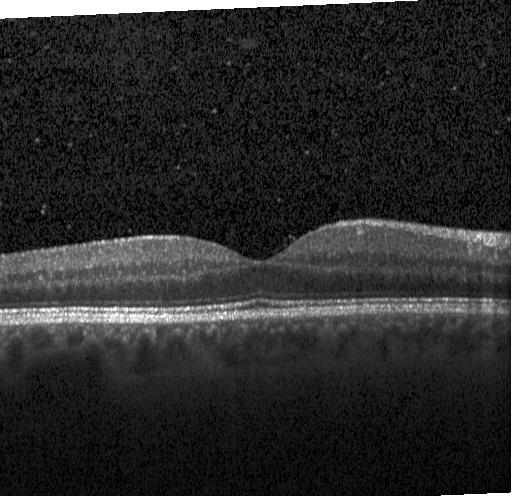
Heidelberg Spectralis OCT system · spectral-domain optical coherence tomography · centered on the fovea · optical coherence tomography B-scan
OCT finding: neither choroidal neovascularization, diabetic macular edema, nor drusen.